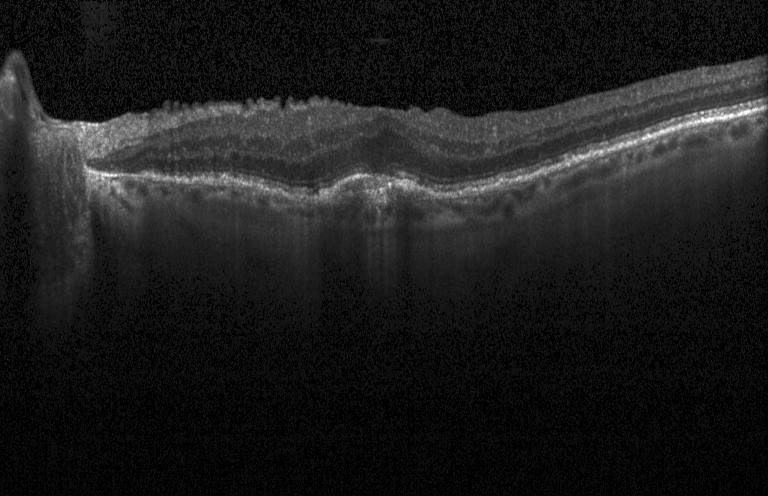

The scan shows choroidal neovascularization.